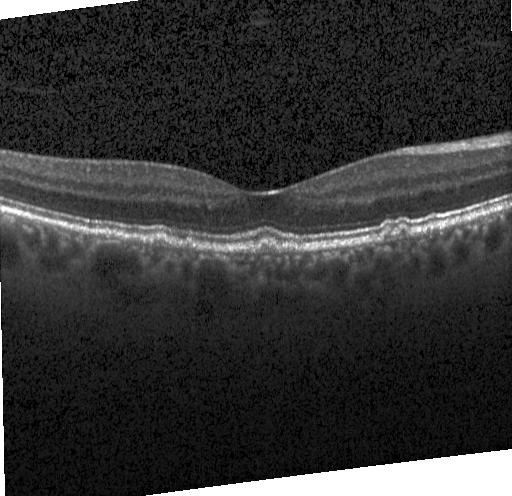 Optical coherence tomography scan
Impression: sub-RPE drusenoid deposits.